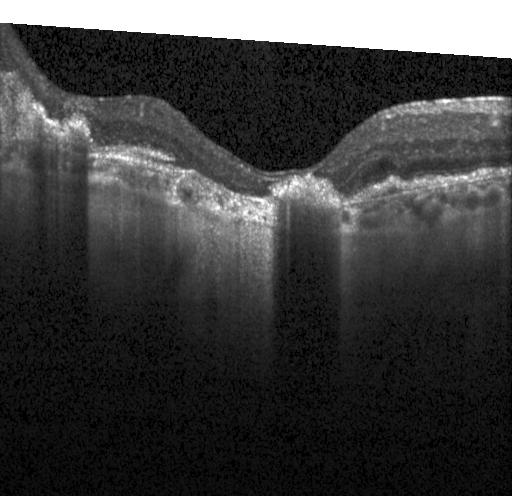 Retinal OCT cross-section
Assessment: choroidal neovascularization.